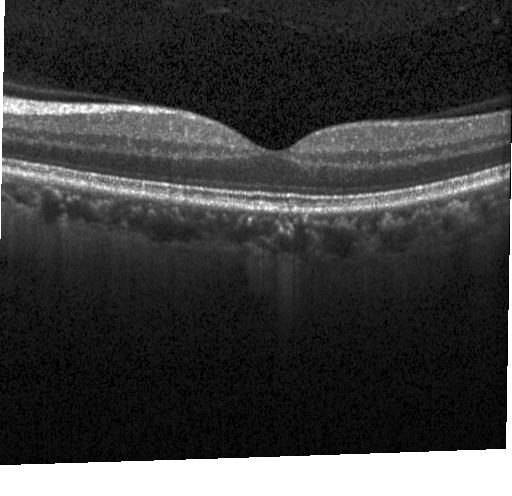 Heidelberg Spectralis OCT system. Optical coherence tomography B-scan.
Diagnosis: no evidence of CNV, DME, or drusen.